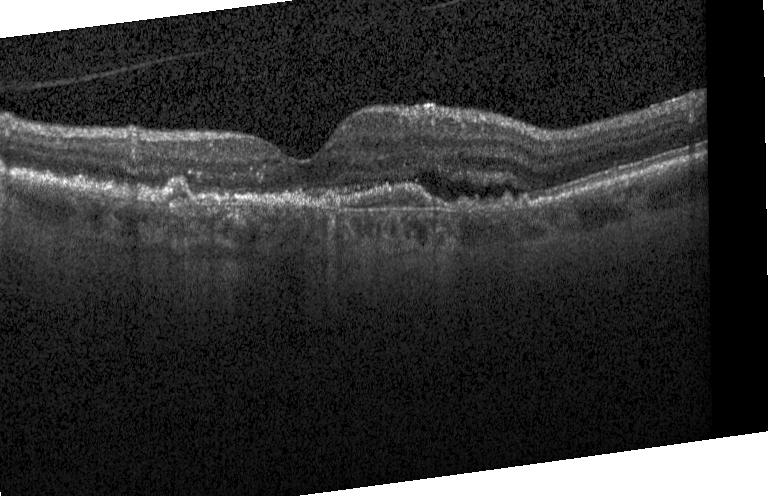 Impression: CNV.